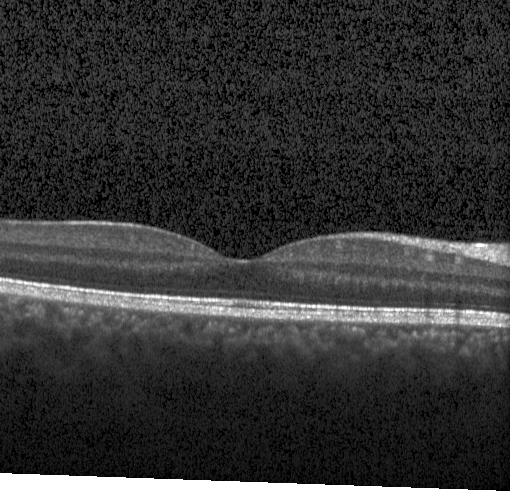 Optical coherence tomography scan.
Impression: no evidence of CNV, DME, or drusen.